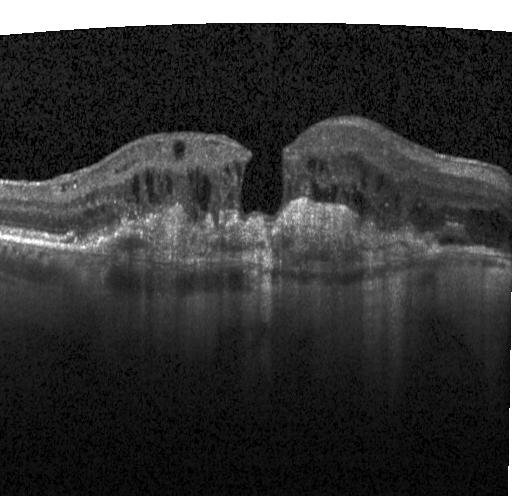
OCT B-scan · SD-OCT.
A choroidal neovascular membrane.